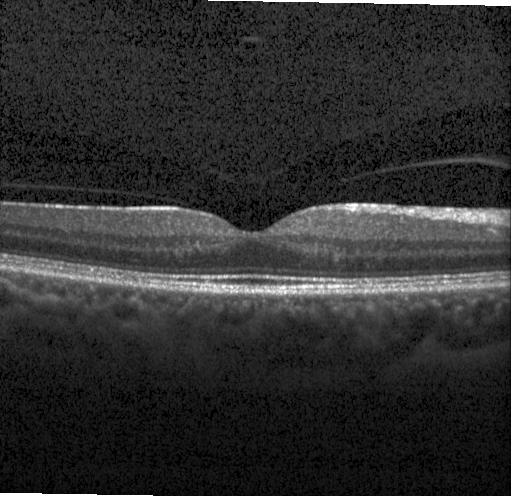

Macular OCT: neither CNV, DME, nor drusen.